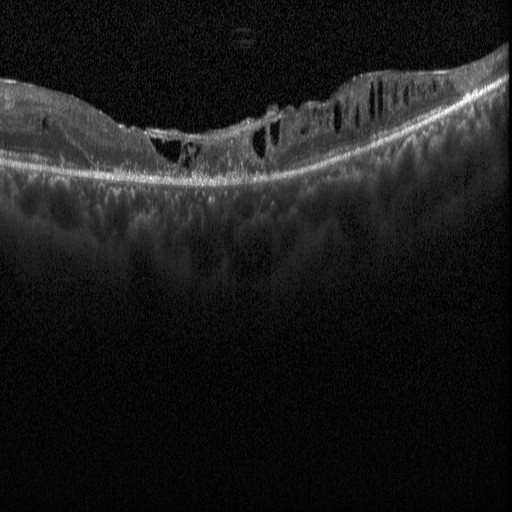 SD-OCT, OCT B-scan.
Diagnosis: DME.